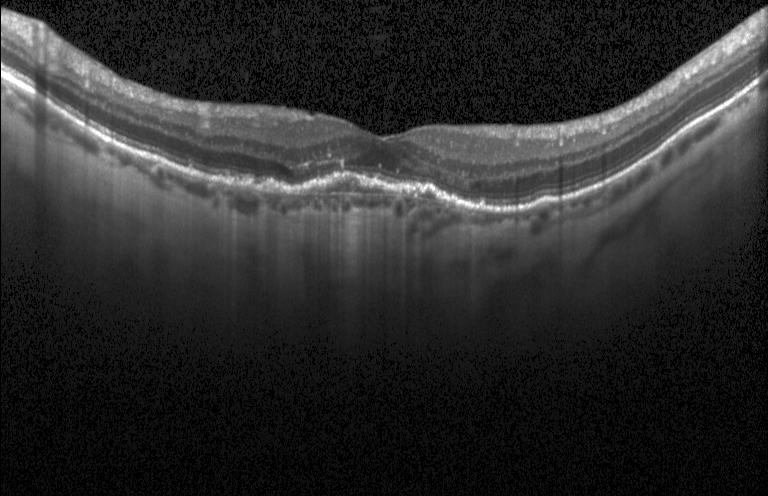 Optical coherence tomography B-scan; SD-OCT
CNV.